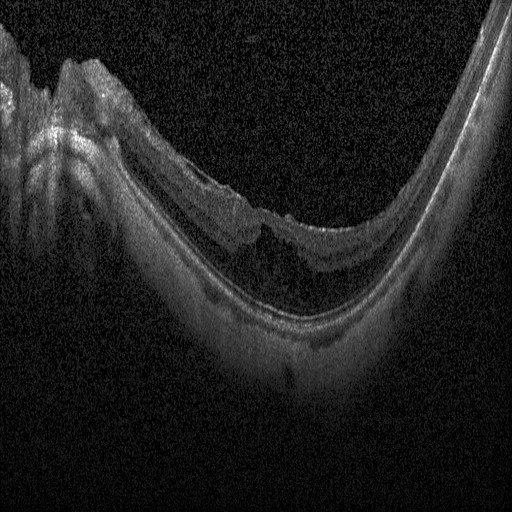

Dx: DME.